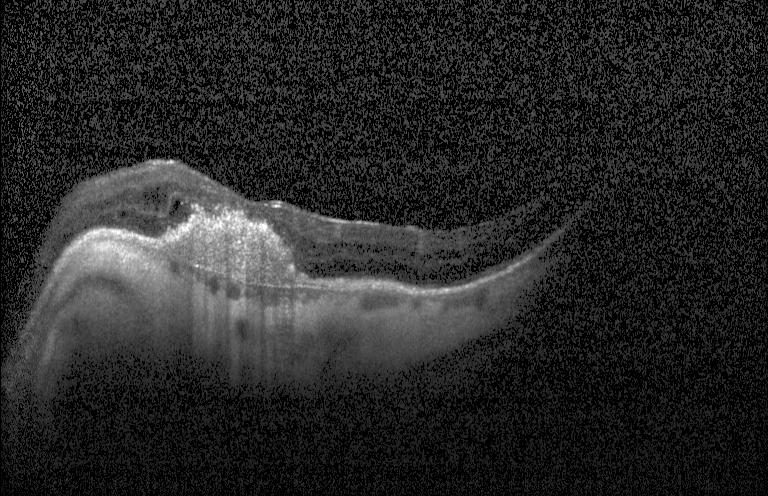

OCT B-scan
Finding: choroidal neovascularization (CNV).